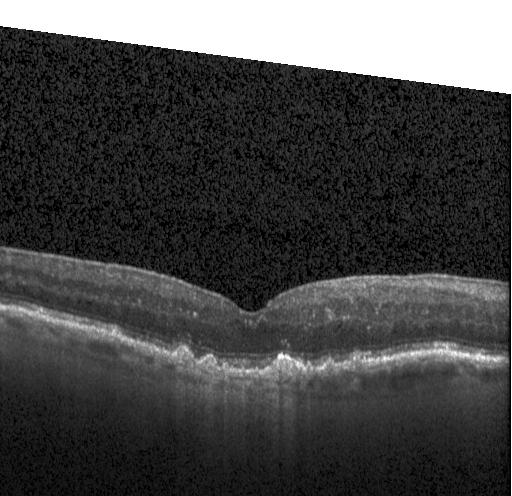 Heidelberg Spectralis, macular scan, spectral-domain optical coherence tomography, retinal OCT B-scan
Diagnosis: CNV.